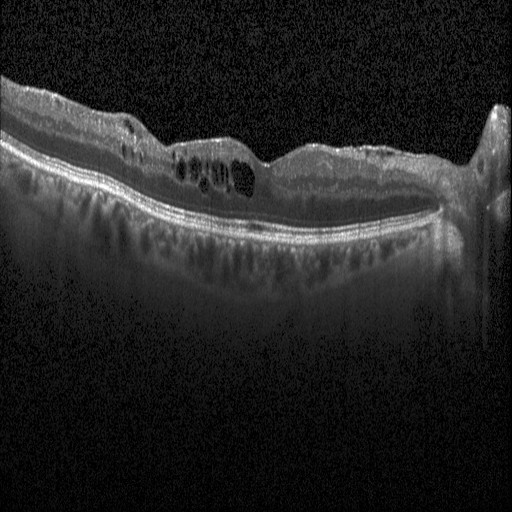
This B-scan demonstrates DME.